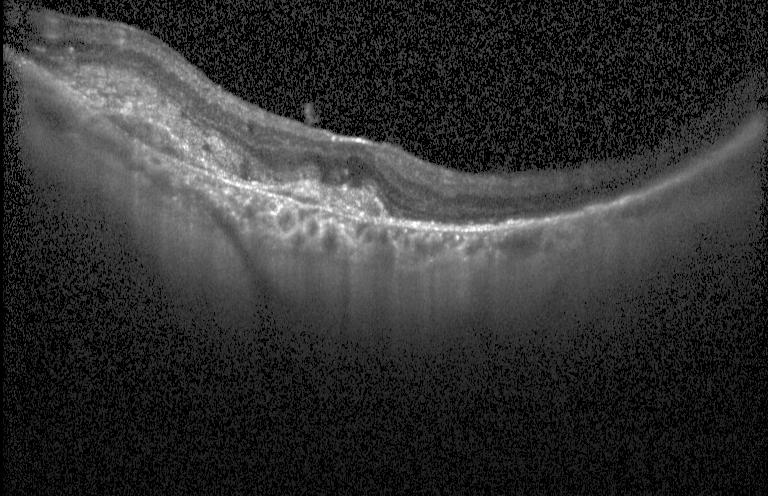

Acquired on a Heidelberg Spectralis; centered on the fovea; retinal OCT cross-section
Impression: a choroidal neovascular membrane.